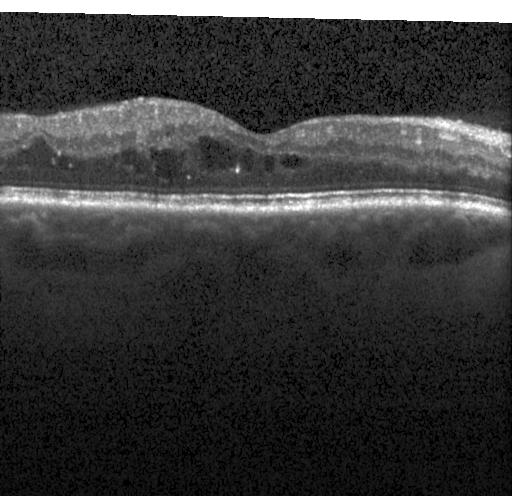 Spectral-domain OCT · acquired on a Heidelberg Spectralis · through the macula · optical coherence tomography scan — This B-scan demonstrates DME.